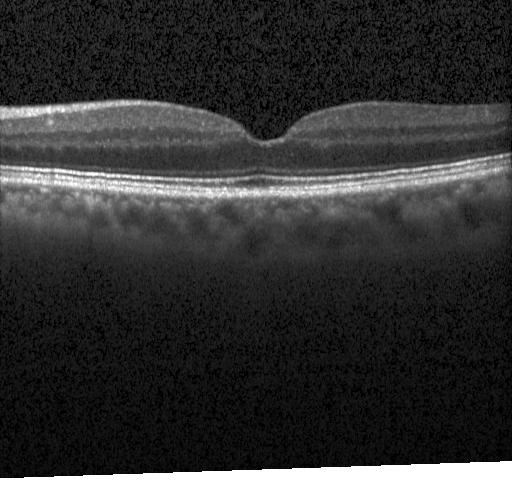

Spectral-domain OCT · fovea-centered · Heidelberg Spectralis OCT system · OCT B-scan.
Macular OCT: no CNV, DME, or drusen.